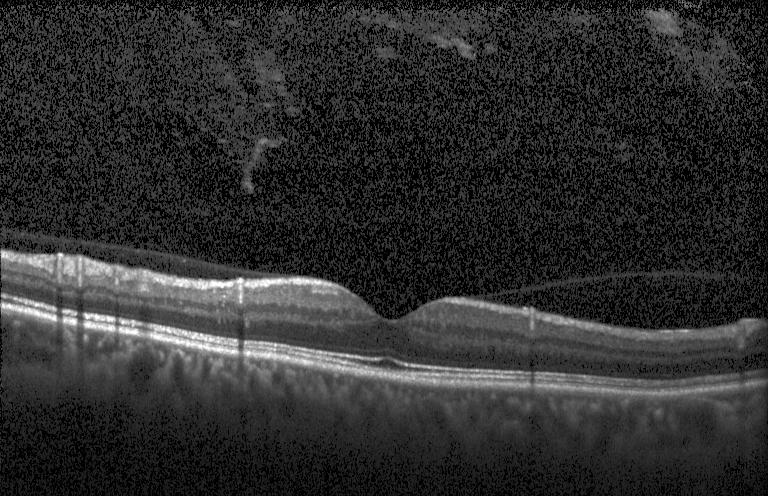
Spectral-domain OCT, instrument: Heidelberg Spectralis, retinal OCT cross-section — OCT finding: neither CNV, DME, nor drusen.